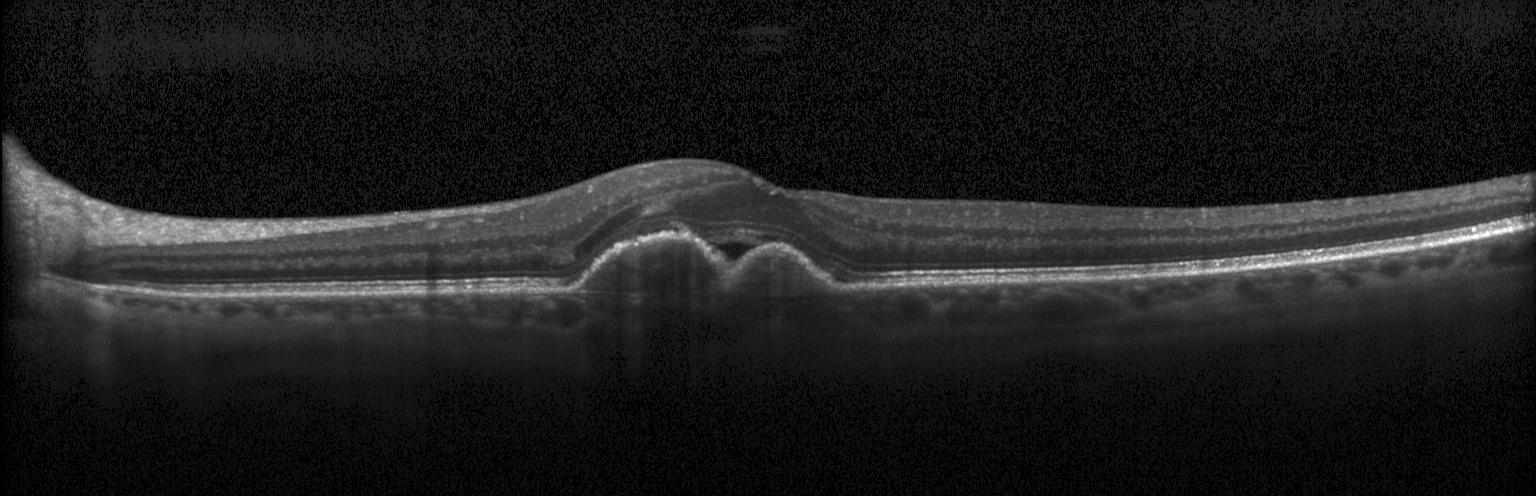 Acquired on a Heidelberg Spectralis; retinal OCT cross-section; spectral-domain OCT. Impression: choroidal neovascularization.